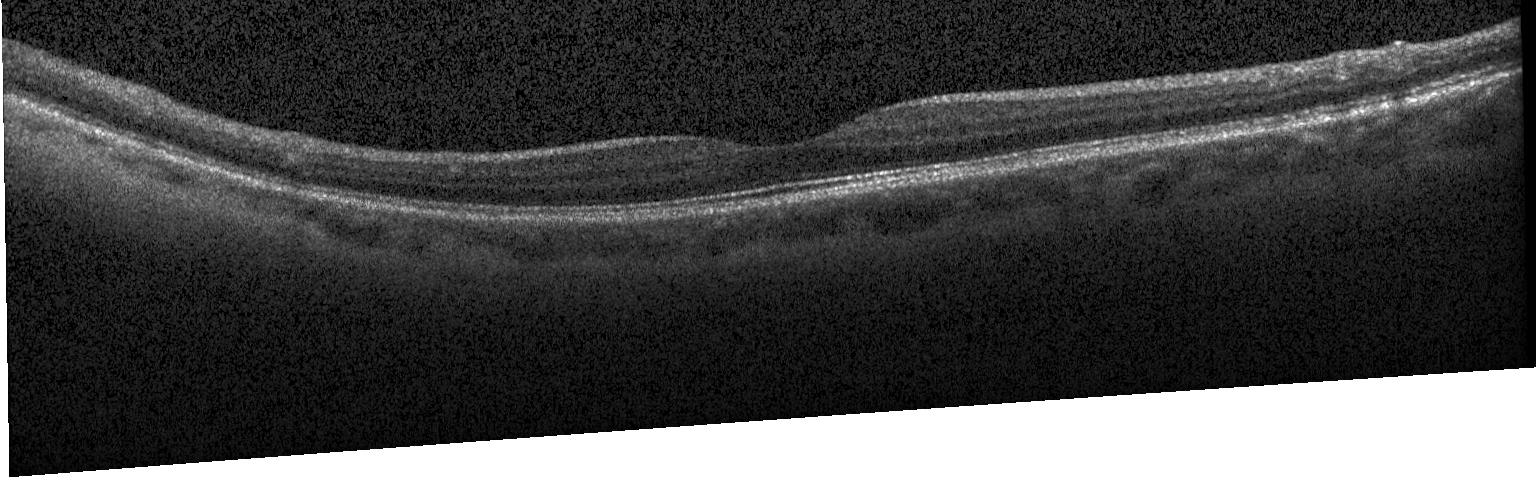 Heidelberg Spectralis, retinal OCT cross-section.
Macular OCT: no evidence of CNV, DME, or drusen.